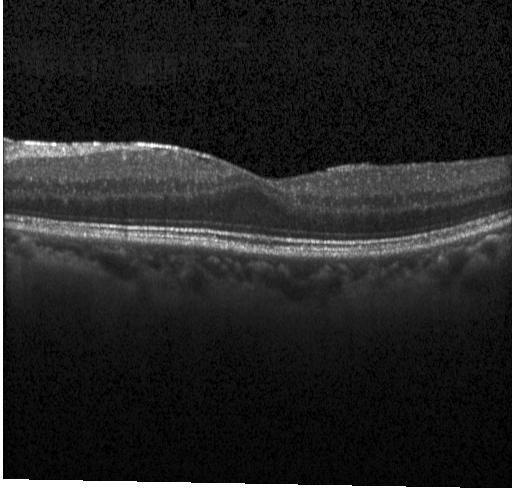 Spectral-domain OCT, Heidelberg Spectralis, OCT B-scan.
The scan shows no CNV, no DME, and no drusen.